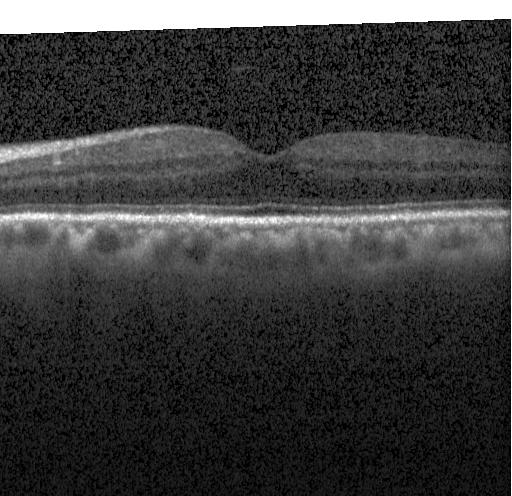 Dx: no evidence of CNV, DME, or drusen.